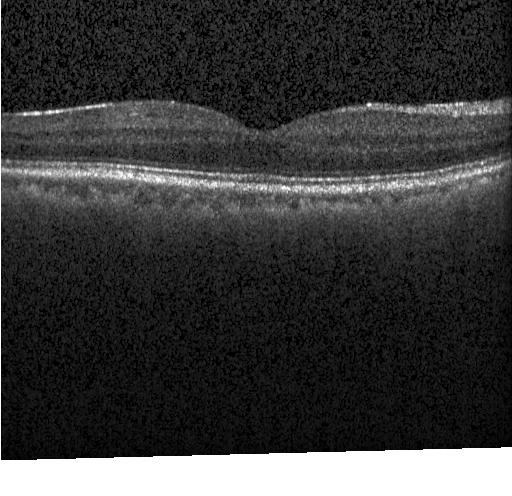
Optical coherence tomography B-scan — Finding: no CNV, DME, or drusen.